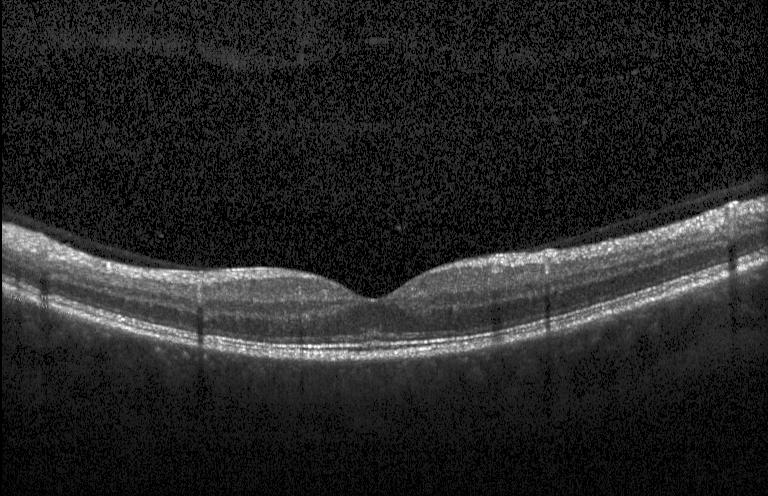

The scan shows no evidence of choroidal neovascularization, diabetic macular edema, or drusen.